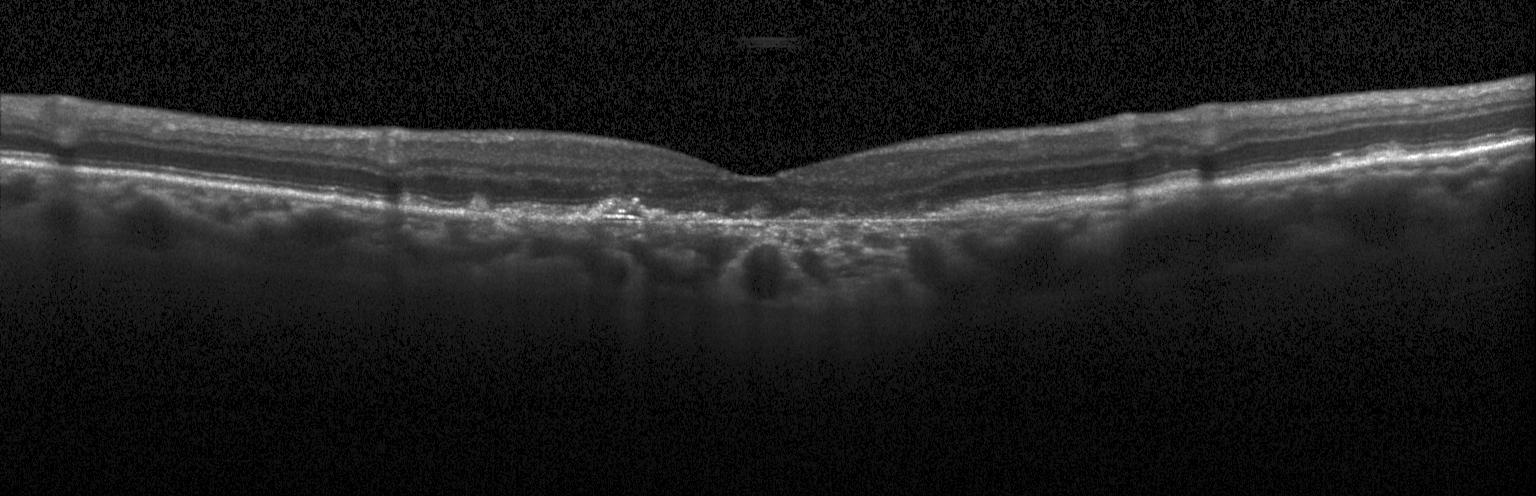

Retinal OCT B-scan, instrument: Heidelberg Spectralis, spectral-domain OCT
Diagnosis: a choroidal neovascular membrane.